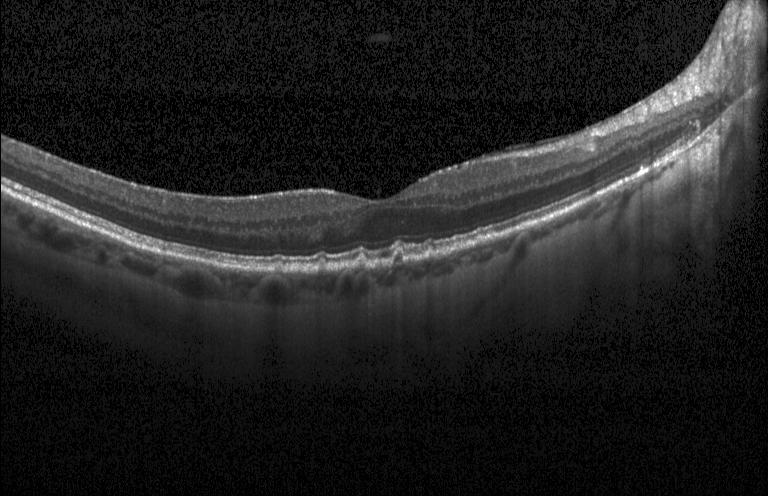

Macular OCT: sub-RPE drusenoid deposits.